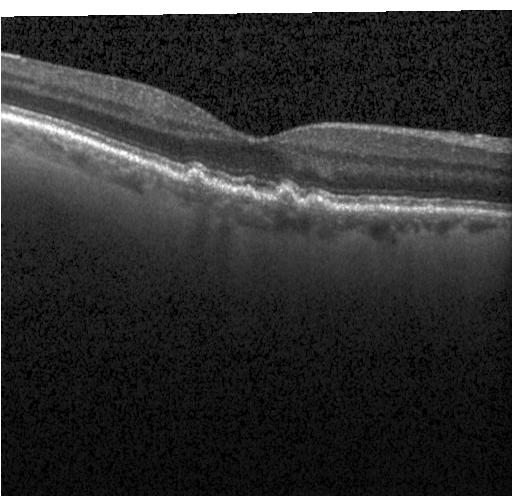
Retinal OCT cross-section showing multiple drusen.